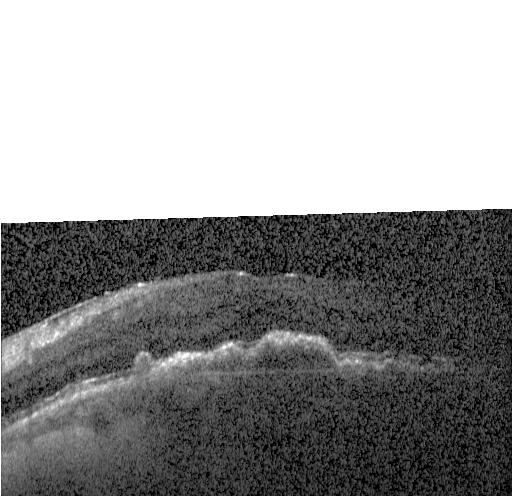
Macular OCT: a choroidal neovascular membrane.